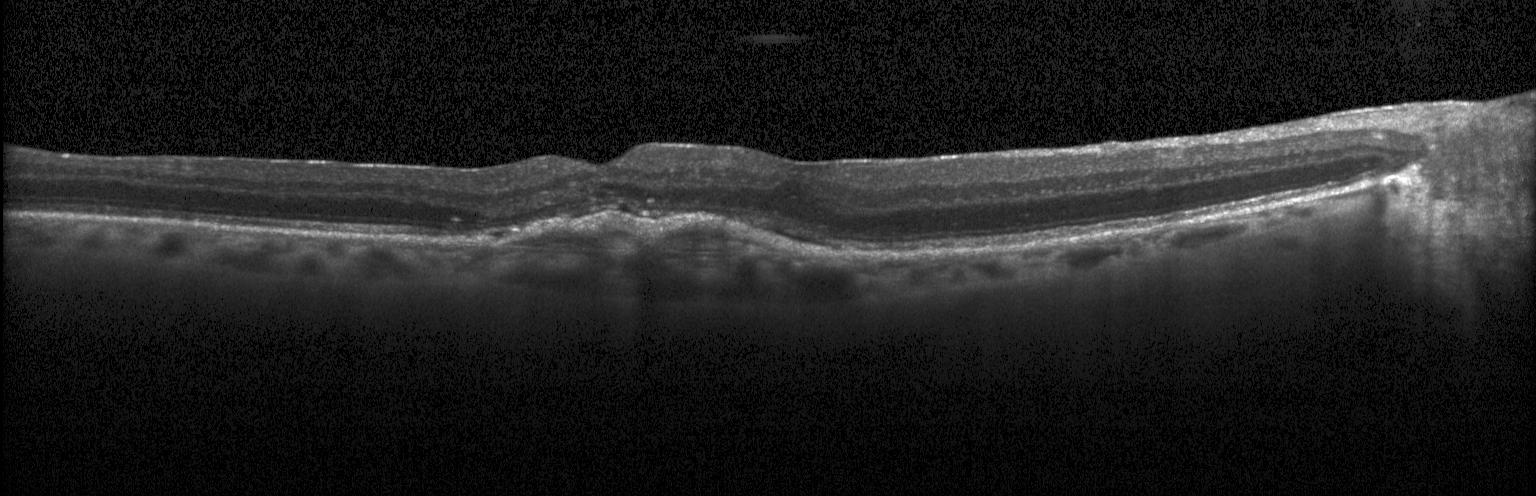

OCT line scan · macular scan. Finding: choroidal neovascularization (CNV).